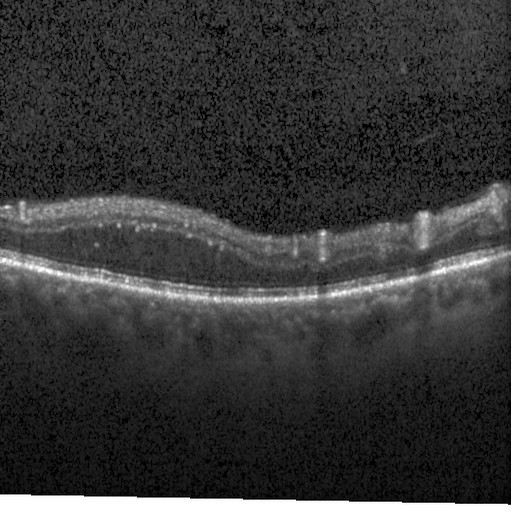
Retinal OCT B-scan — Impression: diabetic macular edema (DME).